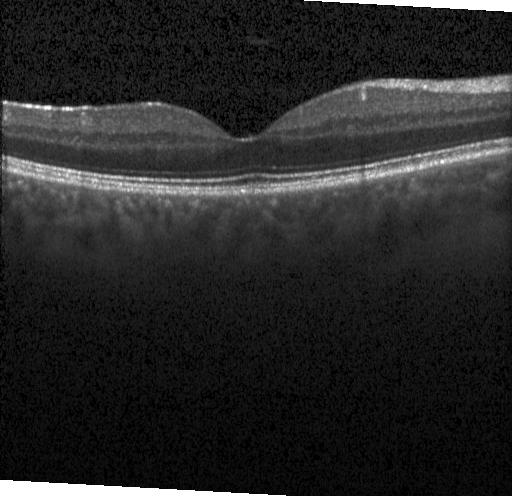
Optical coherence tomography B-scan
Finding: no CNV, DME, or drusen.